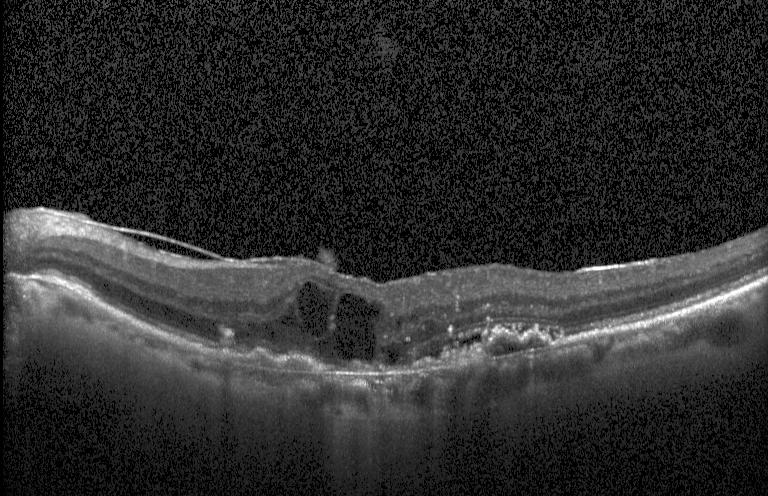 Macular OCT: a choroidal neovascular membrane.